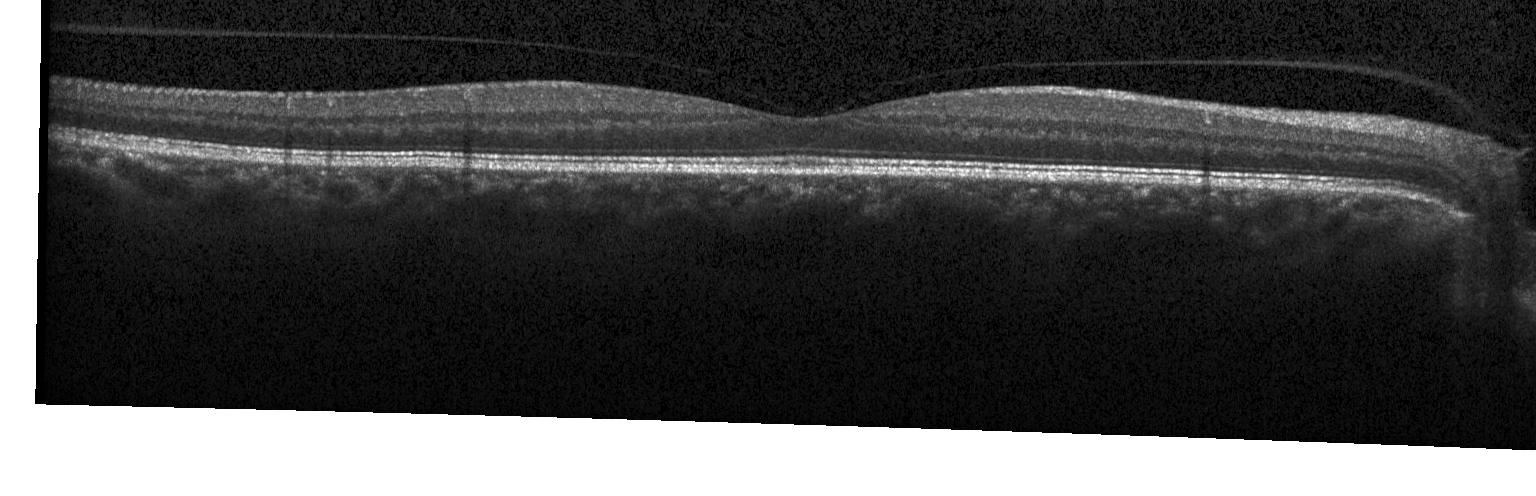 SD-OCT; OCT B-scan; horizontal scan through the fovea
Impression: no choroidal neovascularization, diabetic macular edema, or drusen.